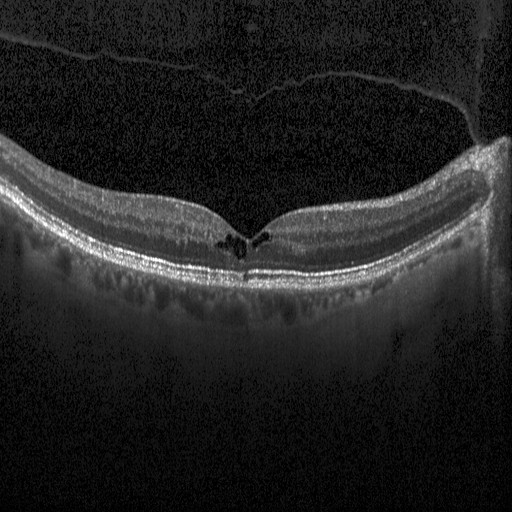
Diagnosis: diabetic macular edema.